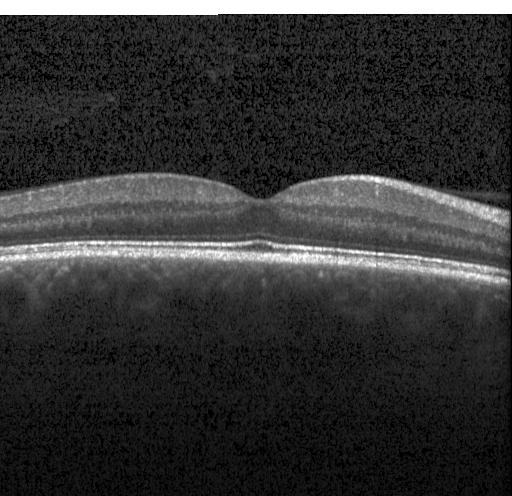 Fovea-centered · OCT B-scan.
Diagnosis: no choroidal neovascularization, diabetic macular edema, or drusen.